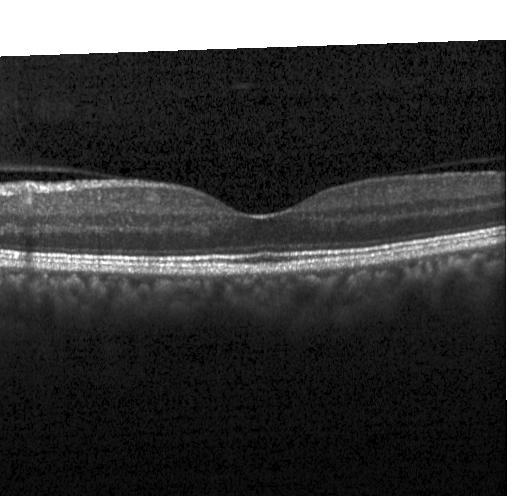

Centered on the fovea, Heidelberg Spectralis, SD-OCT, OCT line scan.
The scan shows no CNV, no DME, and no drusen.